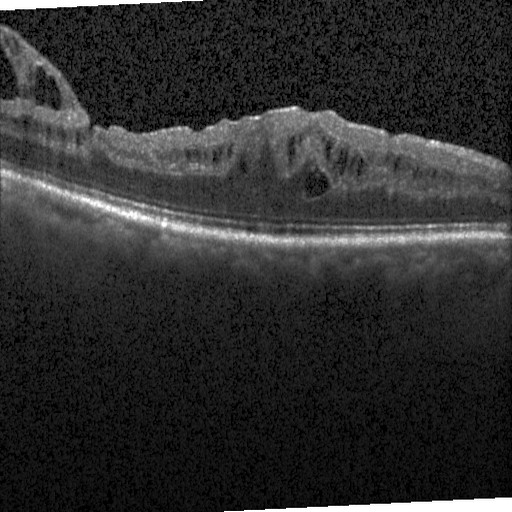 OCT B-scan.
Finding: DME.